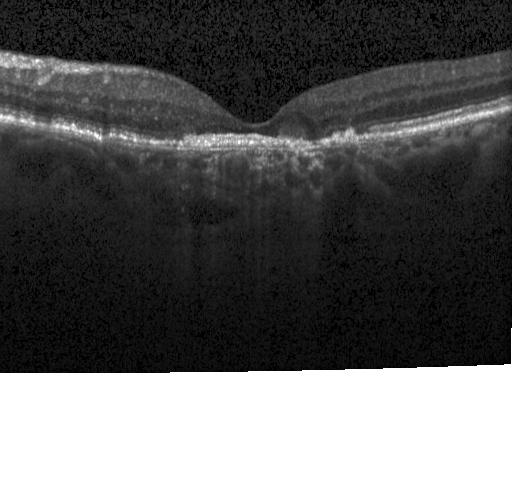 Centered on the fovea, optical coherence tomography scan, spectral-domain optical coherence tomography. Dx: CNV.